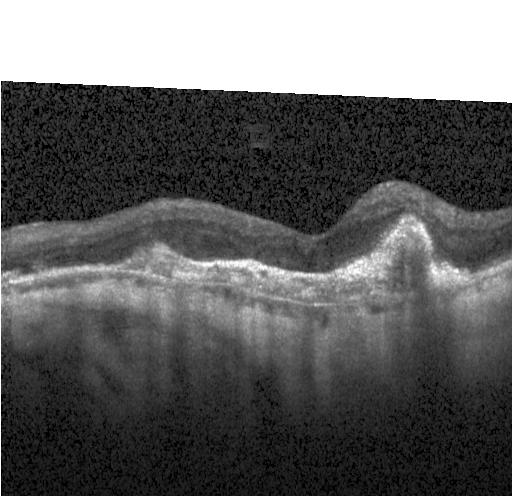

Optical coherence tomography scan
The scan shows a choroidal neovascular membrane.